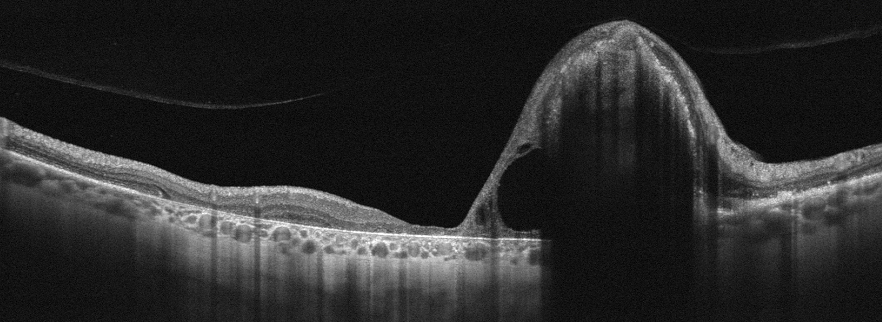

Retinal OCT cross-section
Macular OCT: age-related macular degeneration (AMD).